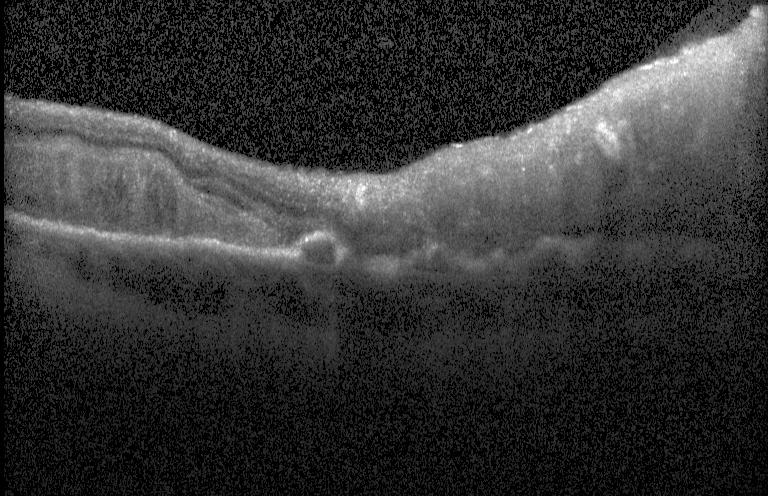

Optical coherence tomography scan
Assessment: a choroidal neovascular membrane.